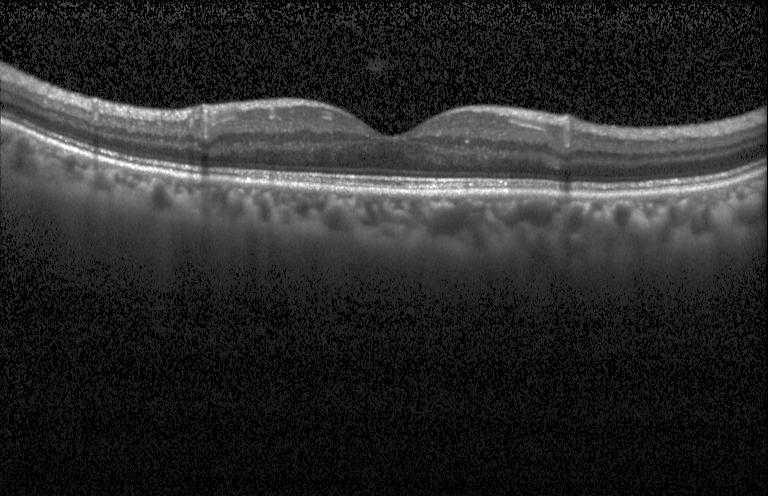 Through the macula, SD-OCT, acquired on a Heidelberg Spectralis, optical coherence tomography B-scan.
Dx: no CNV, no DME, and no drusen.